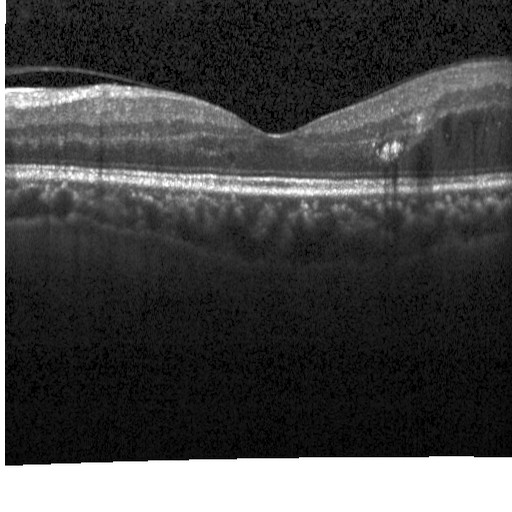

Impression: DME.